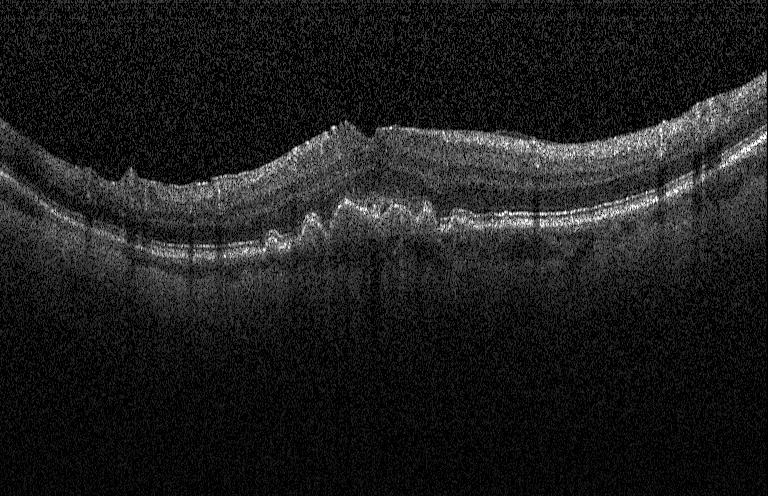
Fovea-centered; spectral-domain optical coherence tomography; optical coherence tomography B-scan — This B-scan demonstrates sub-RPE drusenoid deposits.